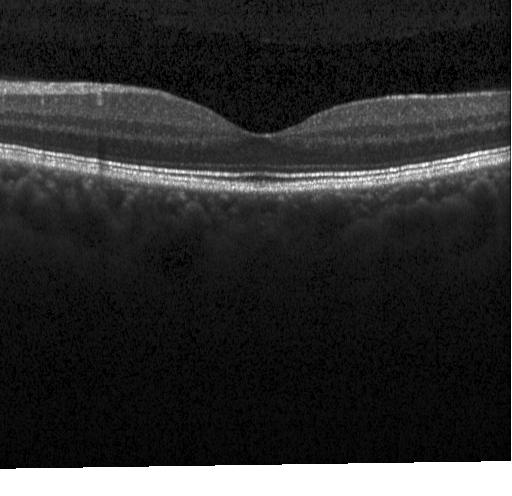 Fovea-centered; acquired on a Heidelberg Spectralis; optical coherence tomography scan; SD-OCT.
Diagnosis: no evidence of choroidal neovascularization, diabetic macular edema, or drusen.